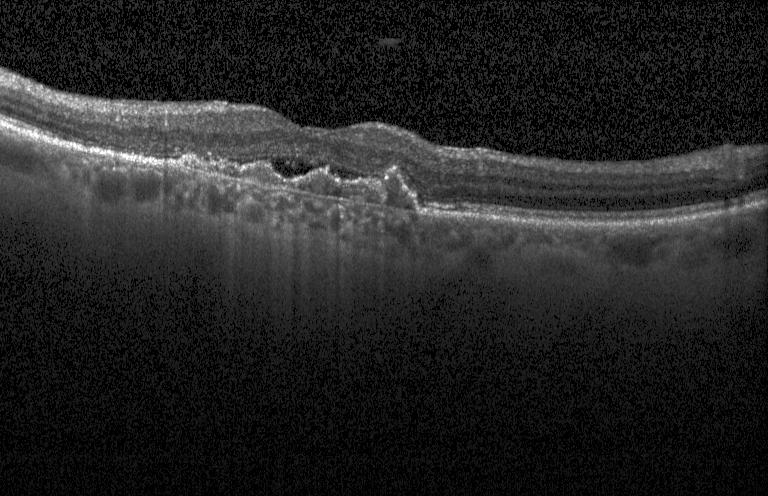 Retinal OCT B-scan, spectral-domain OCT. The scan shows choroidal neovascularization (CNV).